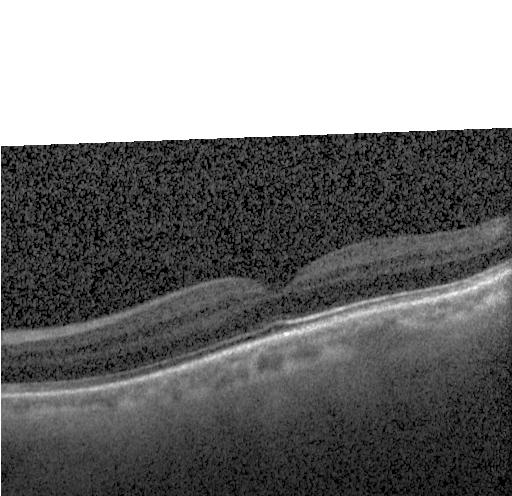

This B-scan demonstrates no evidence of choroidal neovascularization, diabetic macular edema, or drusen.